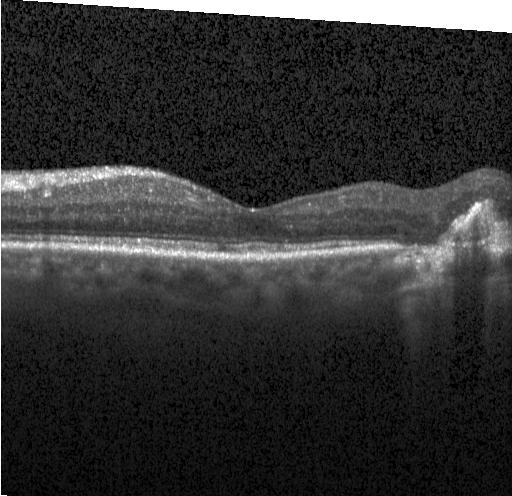

Horizontal scan through the fovea. OCT line scan. Finding: choroidal neovascularization (CNV).